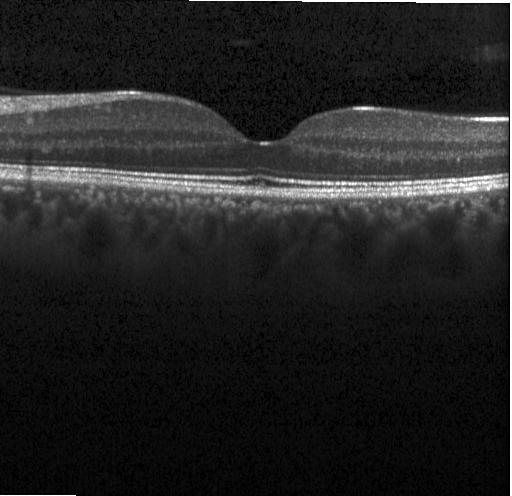

This B-scan demonstrates no CNV, no DME, and no drusen.